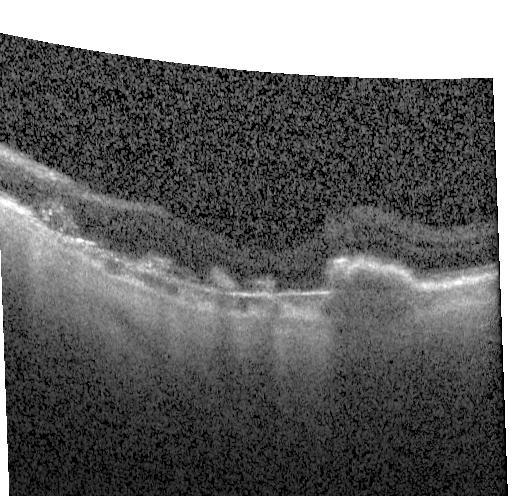
OCT line scan. A choroidal neovascular membrane.